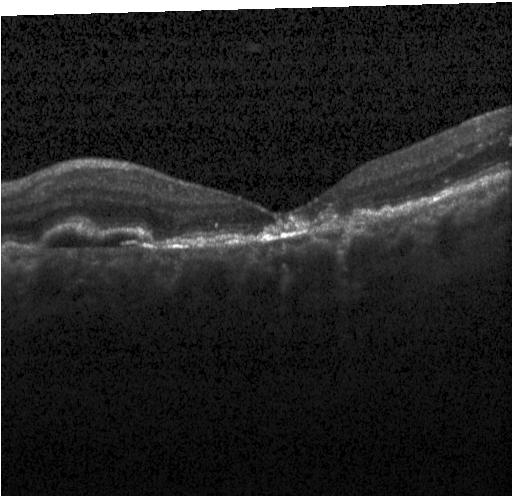
Horizontal scan through the fovea · instrument: Heidelberg Spectralis · OCT line scan. A choroidal neovascular membrane.